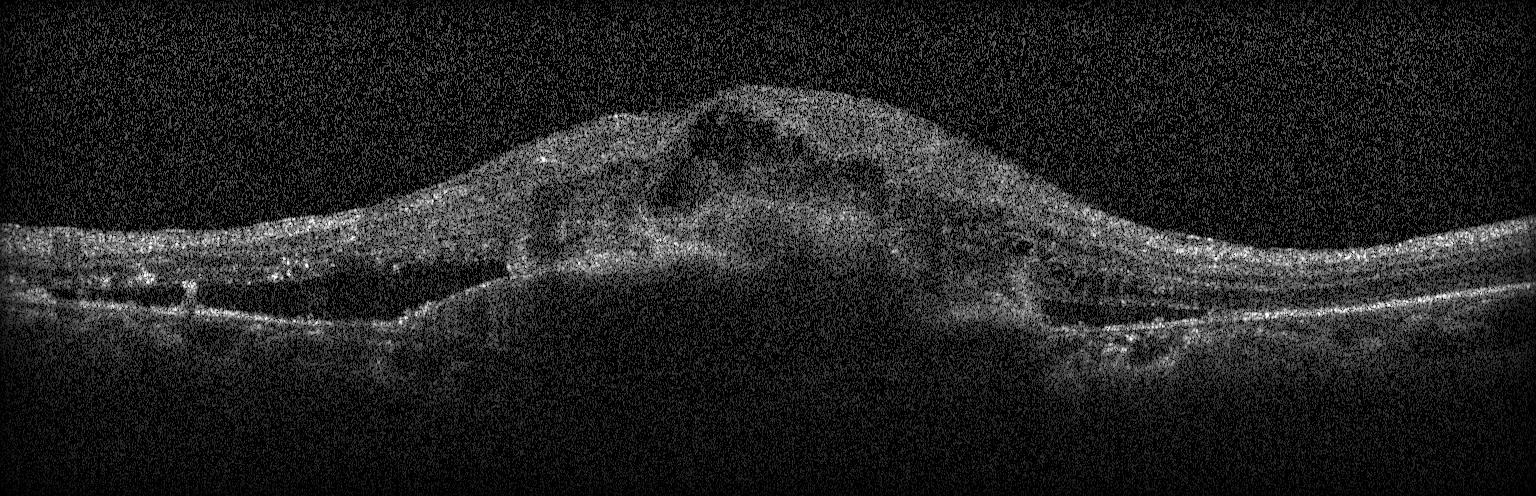 OCT finding: a choroidal neovascular membrane.